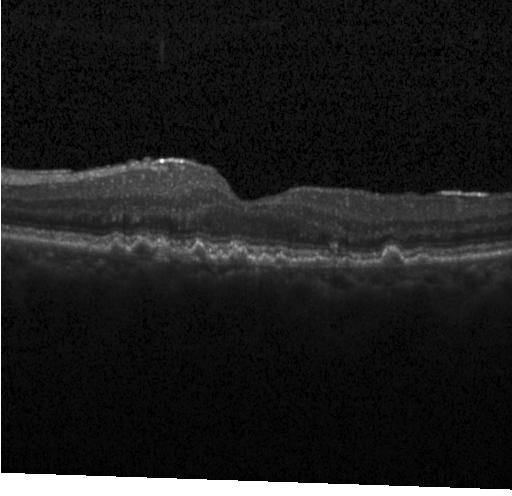 Macular OCT: sub-RPE drusenoid deposits.